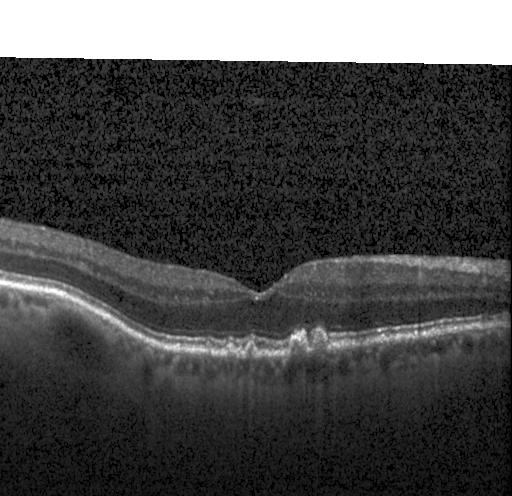
The scan shows multiple drusen.